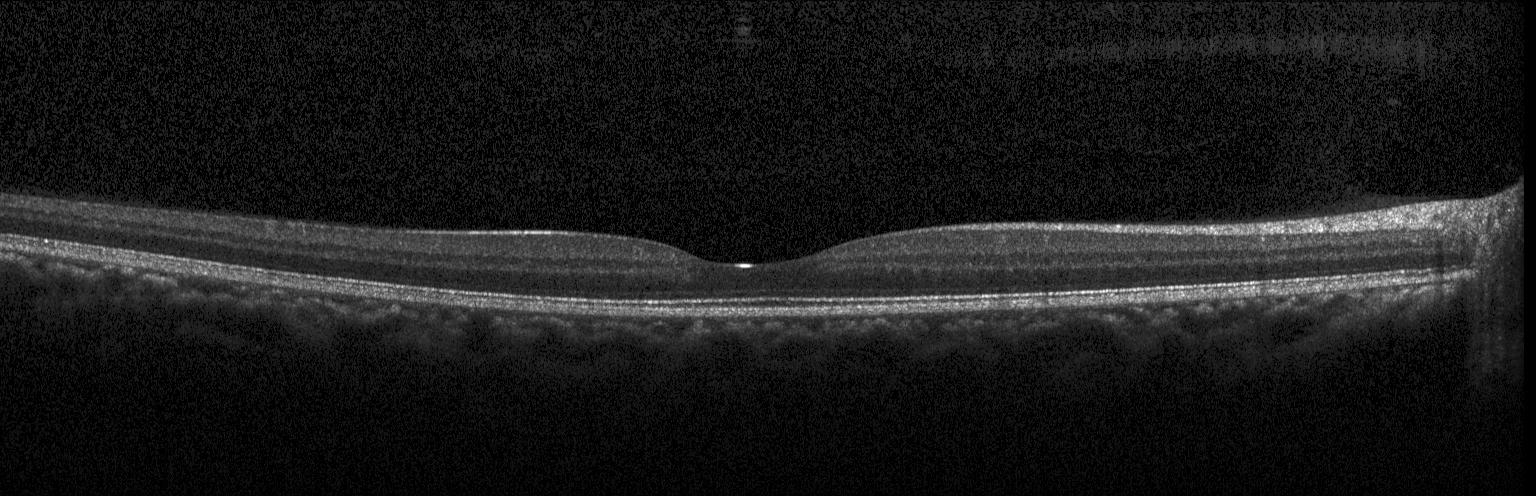 Spectral-domain OCT B-scan: no choroidal neovascularization, diabetic macular edema, or drusen.